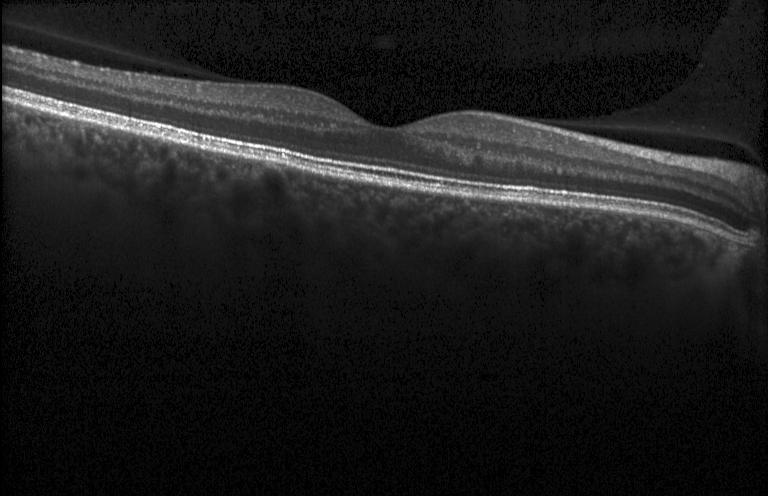
The scan shows neither choroidal neovascularization, diabetic macular edema, nor drusen.